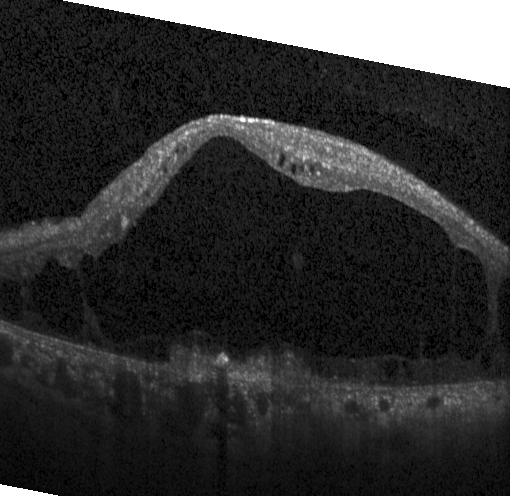 OCT B-scan showing diabetic macular edema (DME).